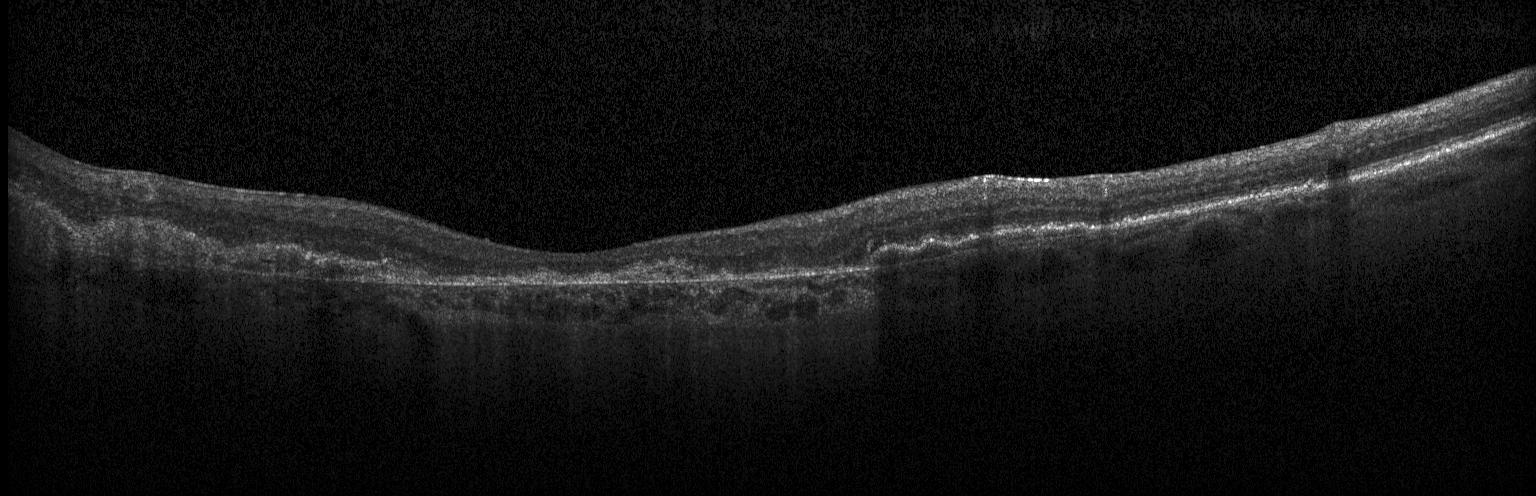 Optical coherence tomography scan
Finding: a choroidal neovascular membrane.